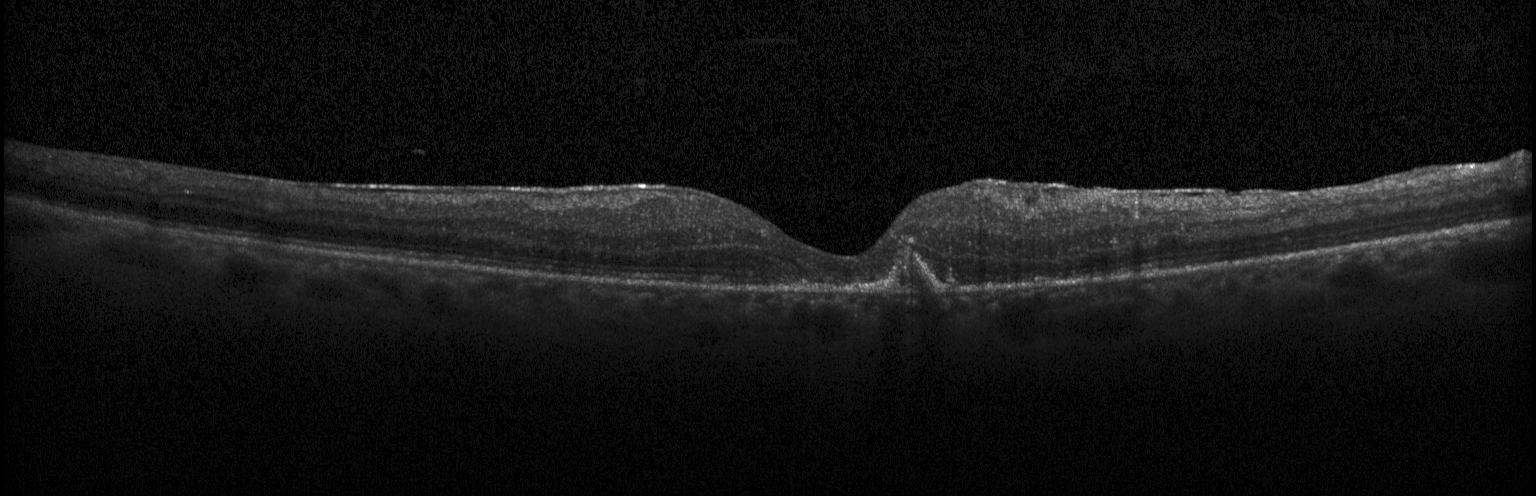 Instrument: Heidelberg Spectralis · optical coherence tomography scan — Finding: a choroidal neovascular membrane.